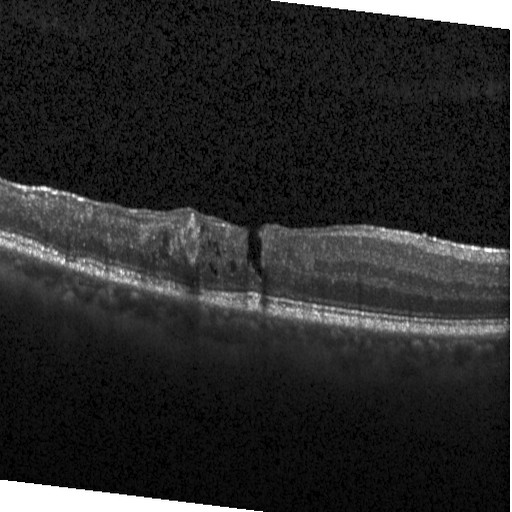 Impression: diabetic macular edema (DME).